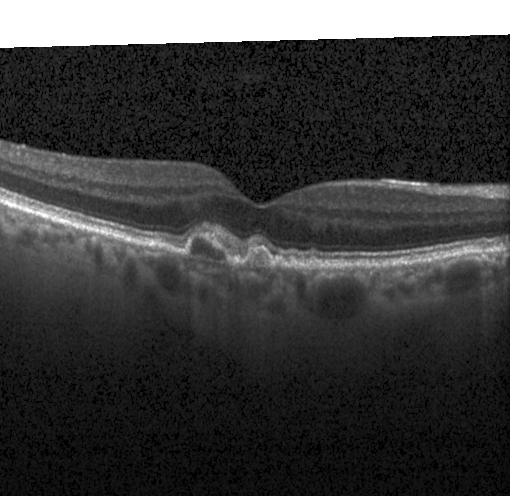
OCT scan showing choroidal neovascularization.